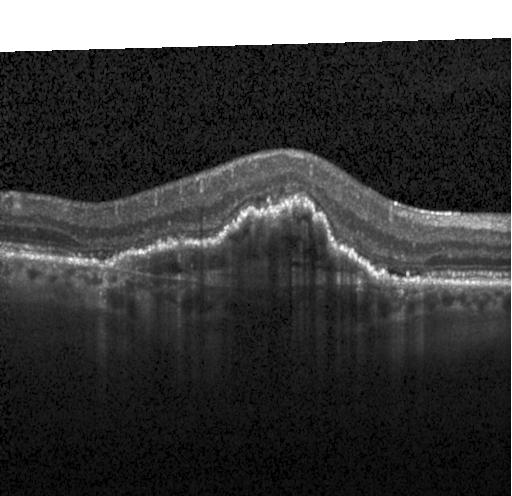
Macular OCT: CNV.